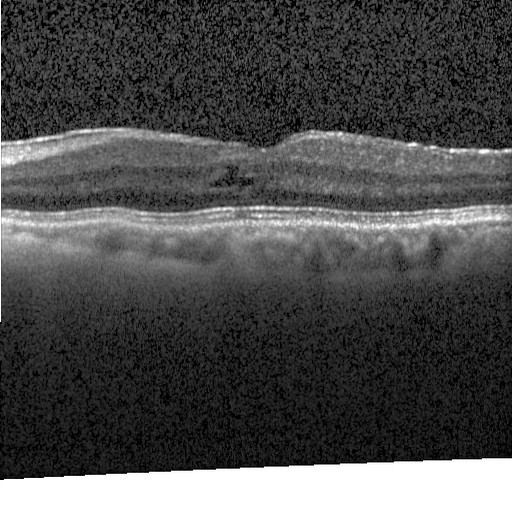

Retinal OCT B-scan.
OCT finding: diabetic macular edema.